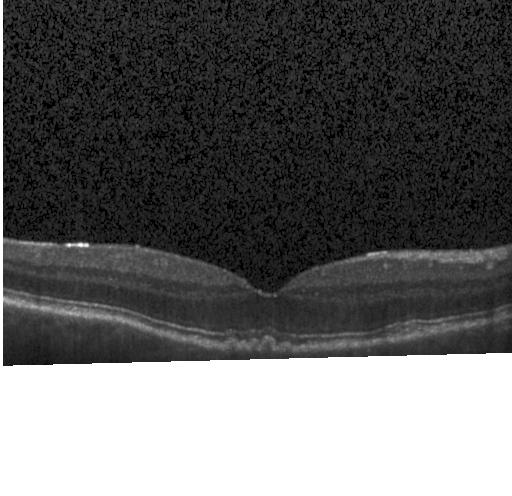
Spectral-domain optical coherence tomography · retinal OCT cross-section · Heidelberg Spectralis OCT system · through the macula.
Macular OCT: multiple drusen.